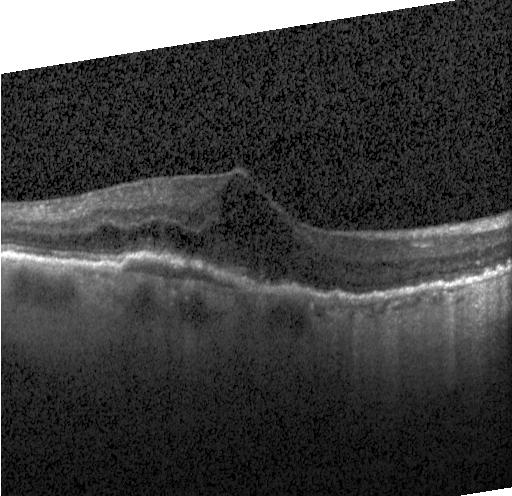

Diagnosis: a choroidal neovascular membrane.